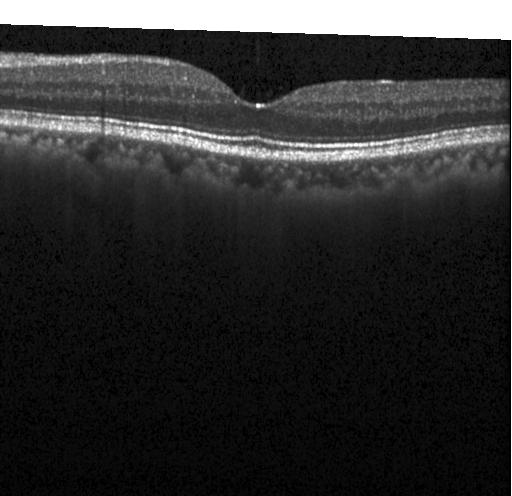

Retinal OCT cross-section. Spectral-domain optical coherence tomography. Macular scan. Instrument: Heidelberg Spectralis — Finding: no choroidal neovascularization, diabetic macular edema, or drusen.